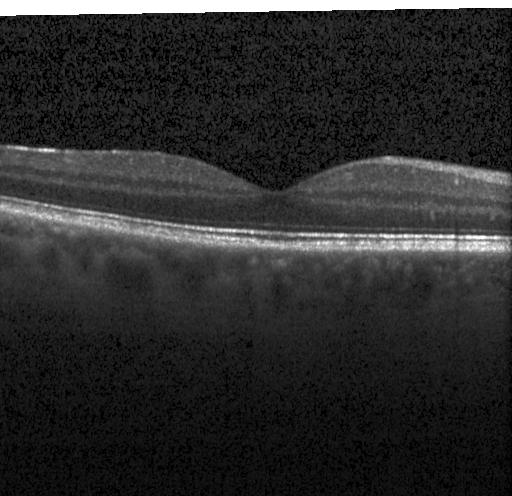

Through the macula; OCT line scan
Impression: no choroidal neovascularization, diabetic macular edema, or drusen.